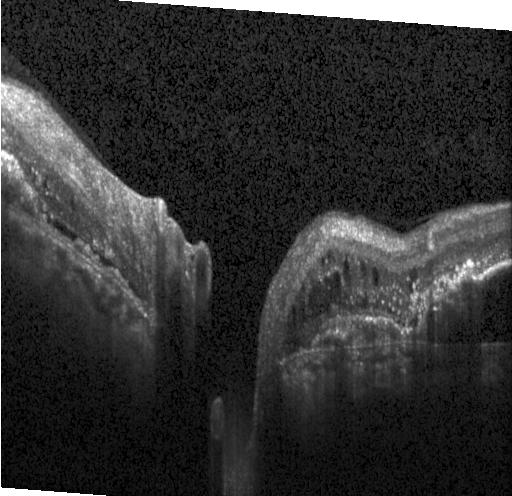
Finding: choroidal neovascularization (CNV).